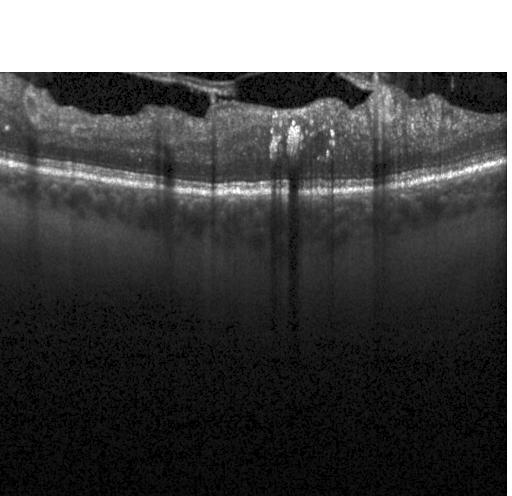

Optical coherence tomography scan. Heidelberg Spectralis OCT system. Spectral-domain OCT. Fovea-centered. Dx: diabetic macular edema (DME).